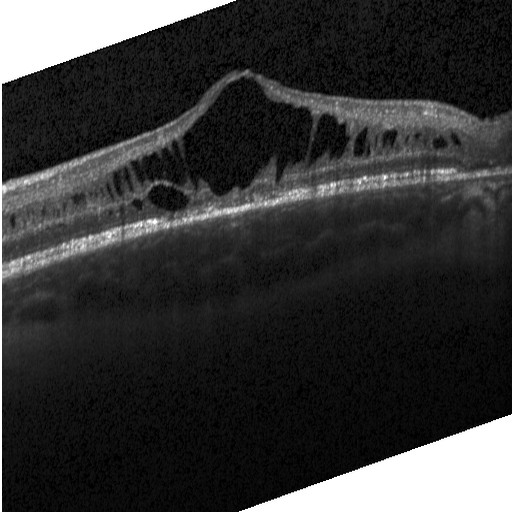 Diagnosis: diabetic macular edema.